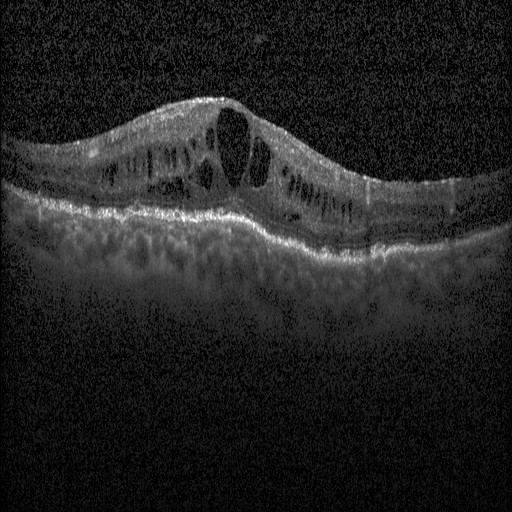

Optical coherence tomography B-scan; SD-OCT. Diagnosis: diabetic macular edema (DME).